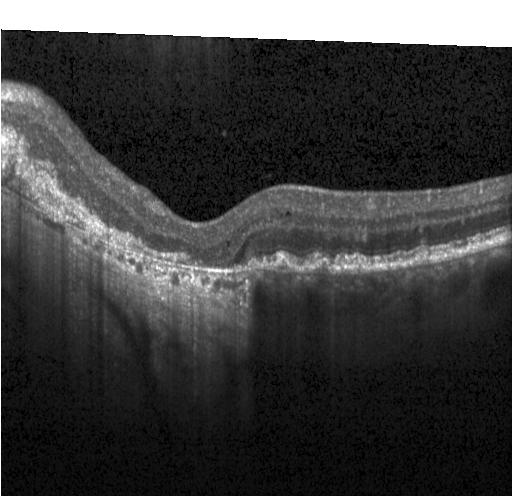 Optical coherence tomography B-scan. Macular scan.
Diagnosis: a choroidal neovascular membrane.